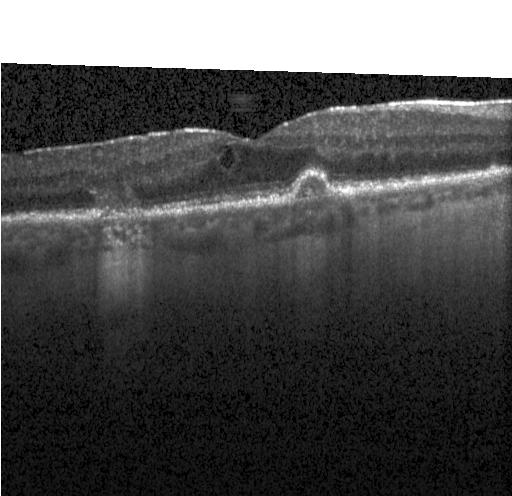 Macular OCT demonstrating diabetic macular edema.